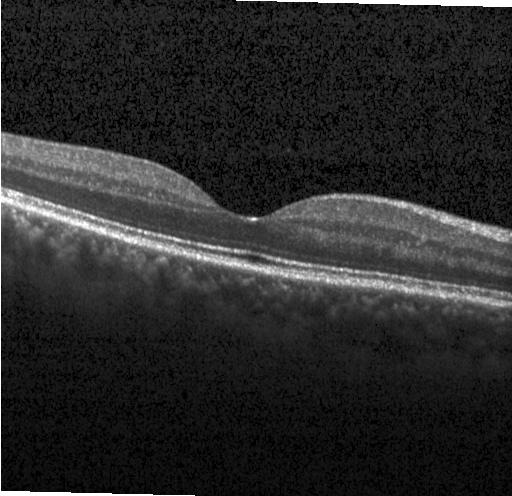
Spectral-domain optical coherence tomography, OCT line scan, Heidelberg Spectralis OCT system, through the macula. No CNV, no DME, and no drusen.